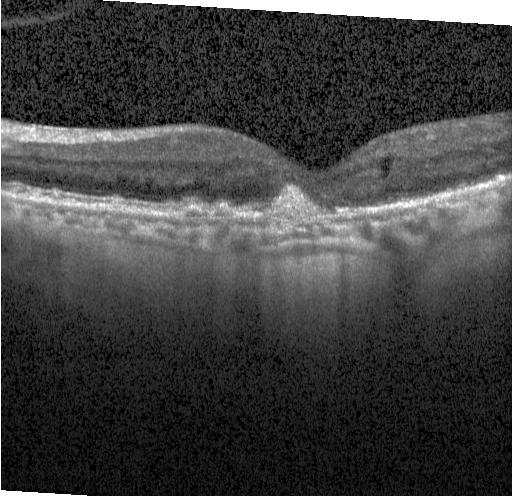
Diagnosis: a choroidal neovascular membrane.